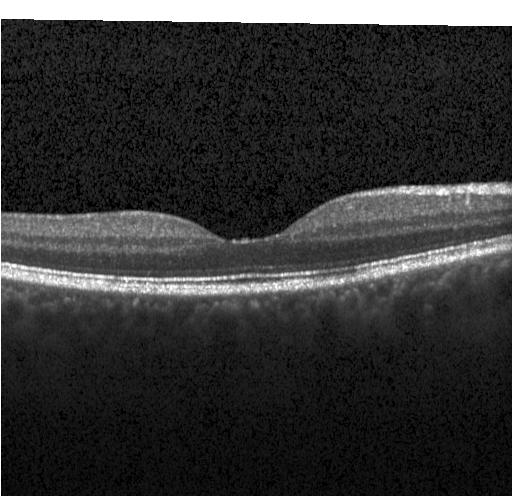
OCT scan showing no choroidal neovascularization, diabetic macular edema, or drusen.